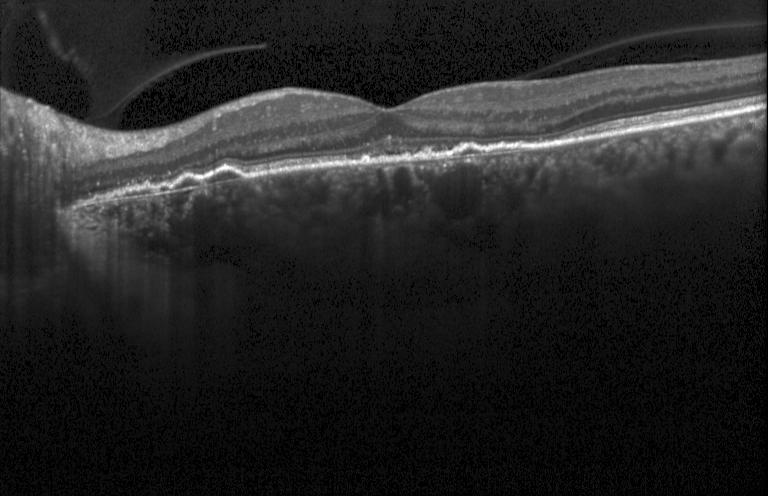

Optical coherence tomography B-scan; Heidelberg Spectralis OCT system; spectral-domain optical coherence tomography. Choroidal neovascularization.